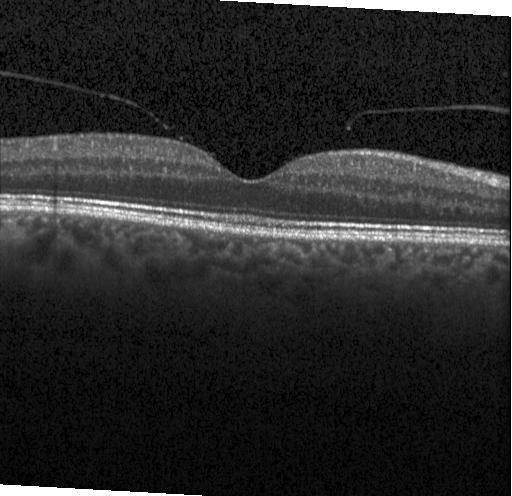
Through the macula · retinal OCT B-scan — The scan shows no choroidal neovascularization, no diabetic macular edema, and no drusen.